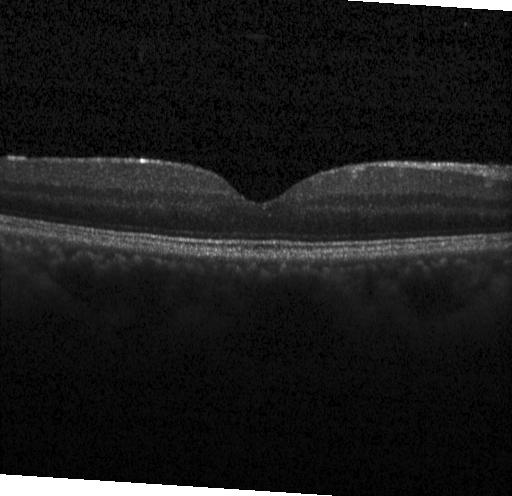 Retinal OCT cross-section · spectral-domain OCT · fovea-centered · instrument: Heidelberg Spectralis. Finding: neither CNV, DME, nor drusen.